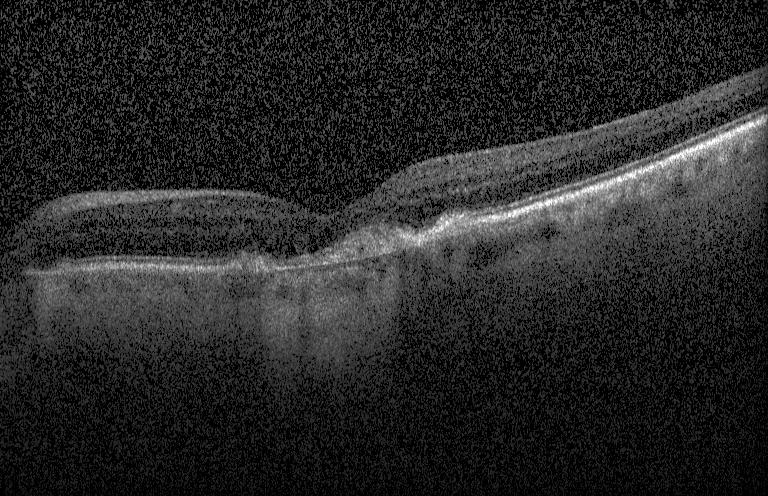 OCT B-scan showing CNV.